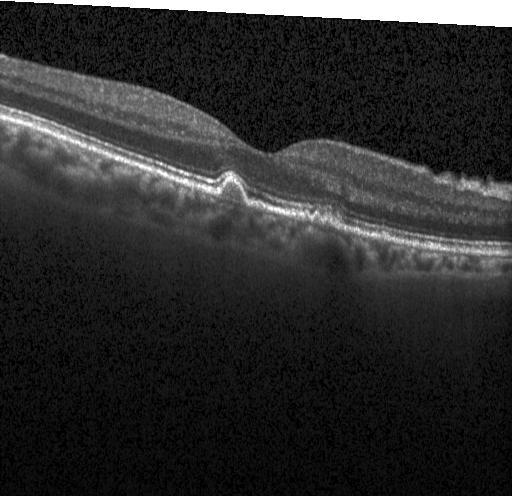

OCT line scan · spectral-domain OCT · fovea-centered — Macular OCT: multiple drusen.